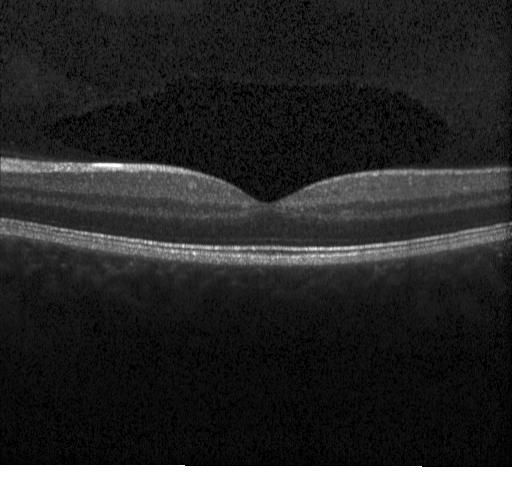

Heidelberg Spectralis OCT system; OCT line scan; through the macula; spectral-domain optical coherence tomography
Assessment: no evidence of choroidal neovascularization, diabetic macular edema, or drusen.